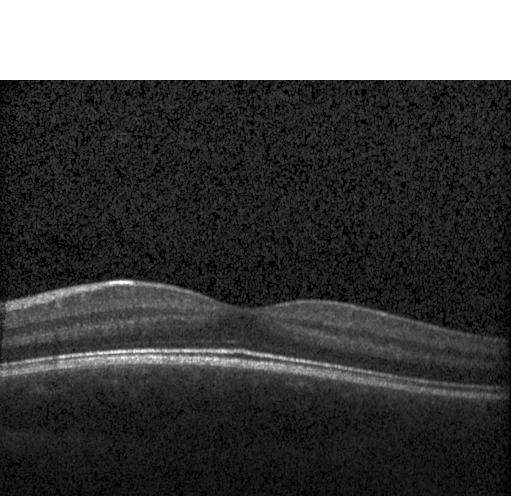 Finding: no choroidal neovascularization, no diabetic macular edema, and no drusen.